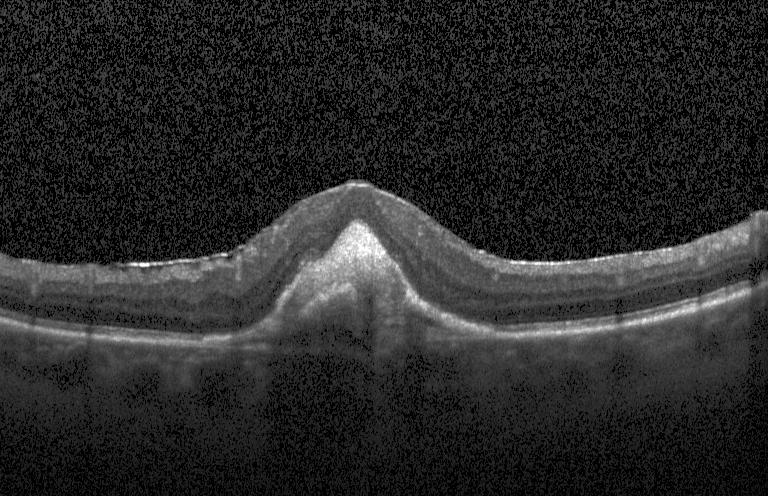 Spectral-domain optical coherence tomography · Heidelberg Spectralis OCT system · retinal OCT cross-section · through the macula.
Macular OCT: CNV.